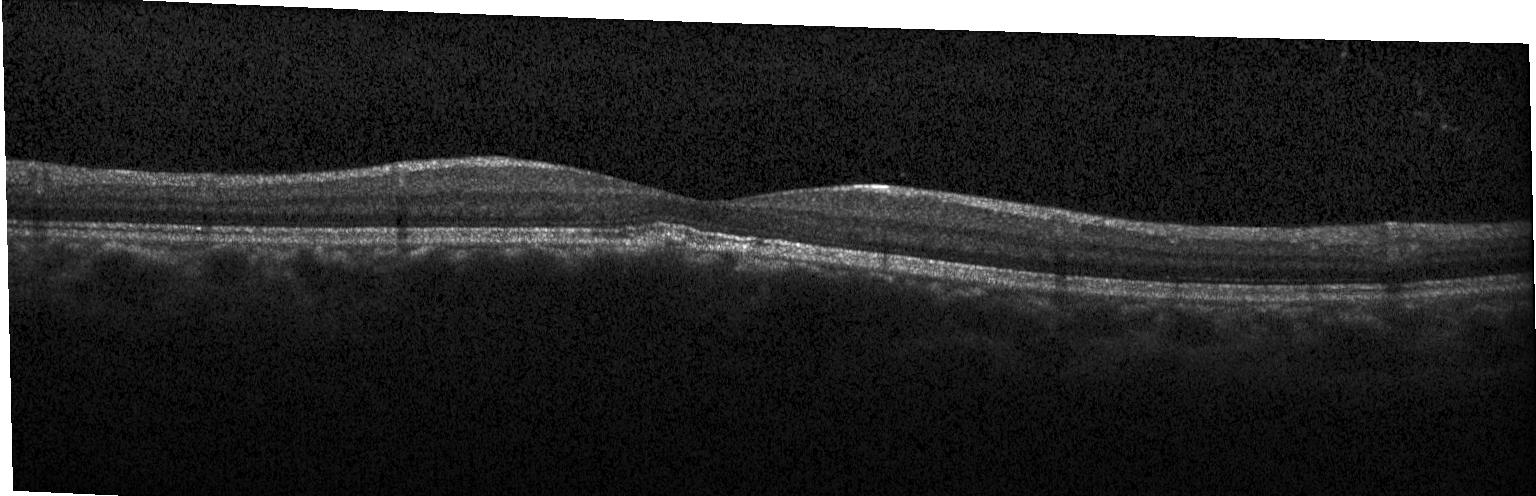
Optical coherence tomography B-scan. Heidelberg Spectralis
Finding: multiple drusen.